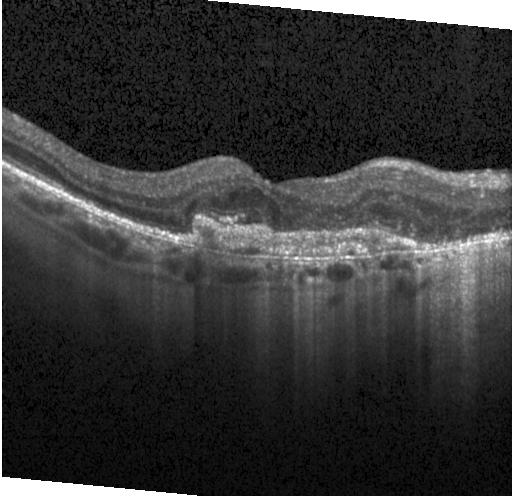

Centered on the fovea; retinal OCT B-scan; acquired on a Heidelberg Spectralis; spectral-domain optical coherence tomography — Choroidal neovascularization.